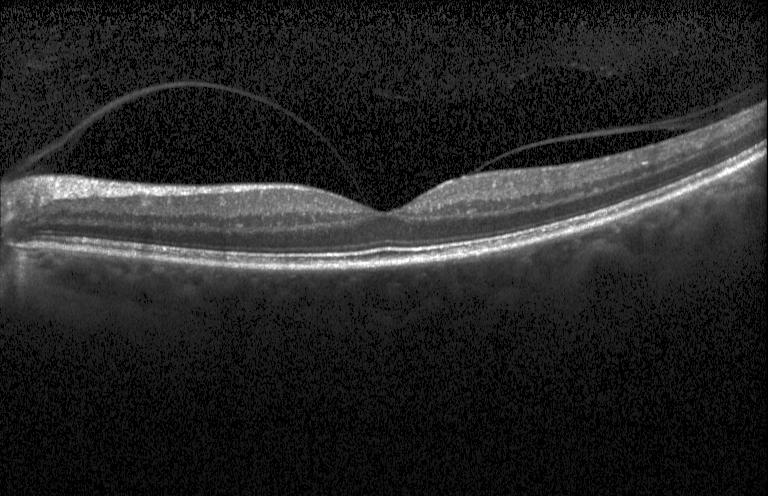 The scan shows neither choroidal neovascularization, diabetic macular edema, nor drusen.